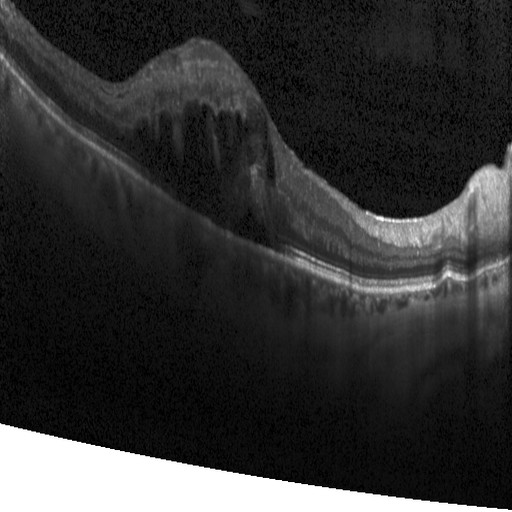

OCT finding: DME.